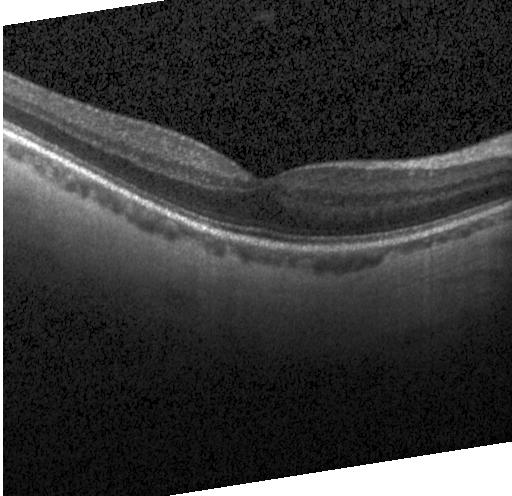 Diagnosis: neither CNV, DME, nor drusen.